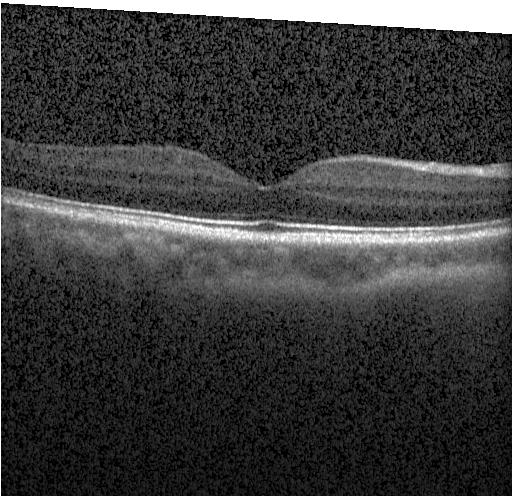

Macular scan; optical coherence tomography scan. The scan shows no choroidal neovascularization, diabetic macular edema, or drusen.